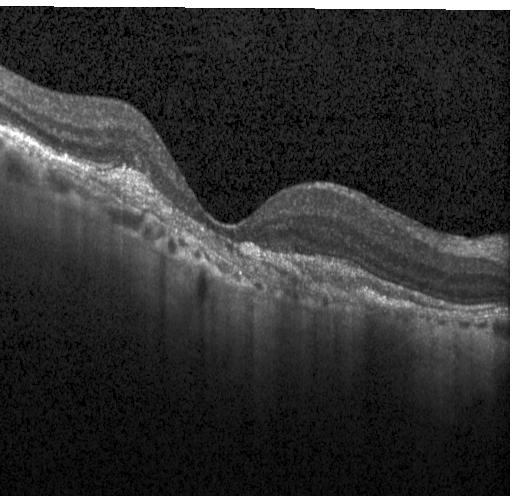
Retinal OCT B-scan; Heidelberg Spectralis; macular scan. Impression: CNV.